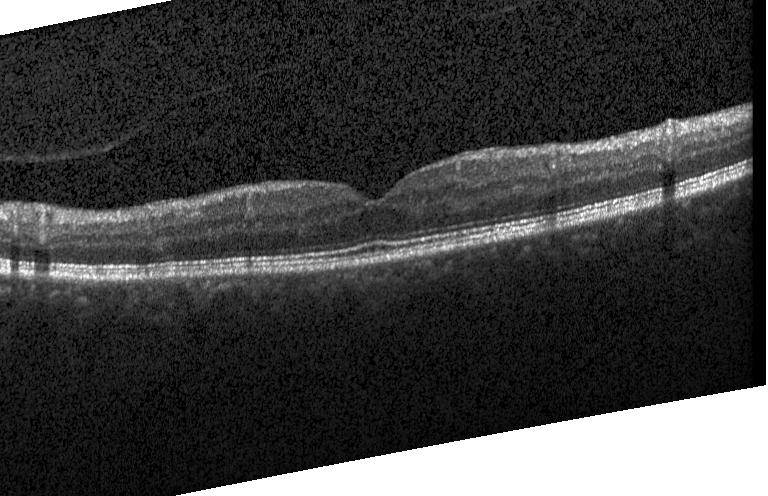 Retinal OCT B-scan
Neither choroidal neovascularization, diabetic macular edema, nor drusen.